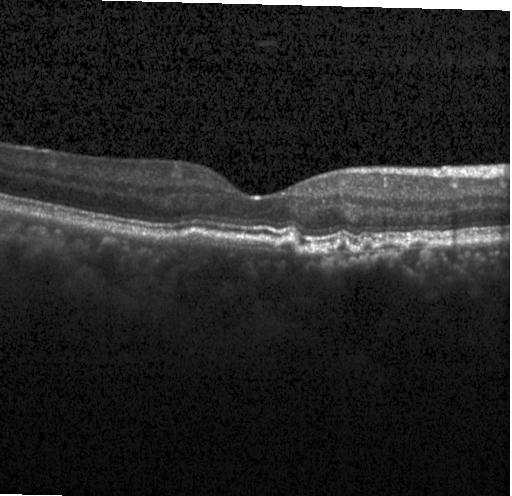 Spectral-domain optical coherence tomography; through the macula; OCT line scan
This B-scan demonstrates drusen.